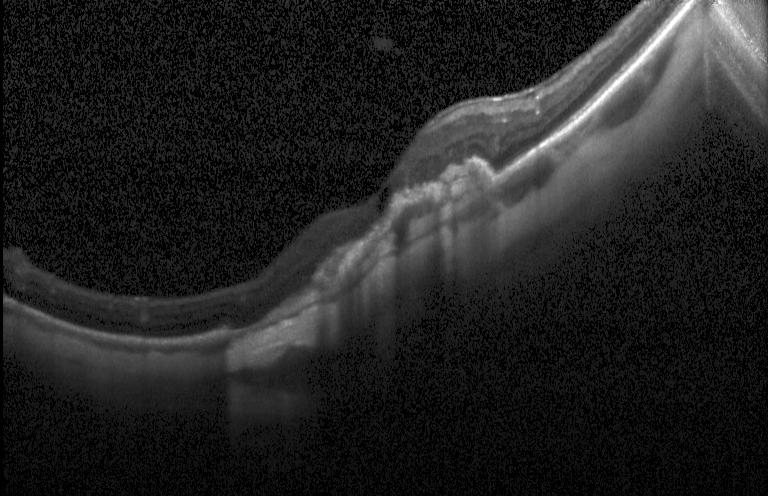 Spectral-domain OCT, OCT B-scan, macular scan — Macular OCT: choroidal neovascularization.